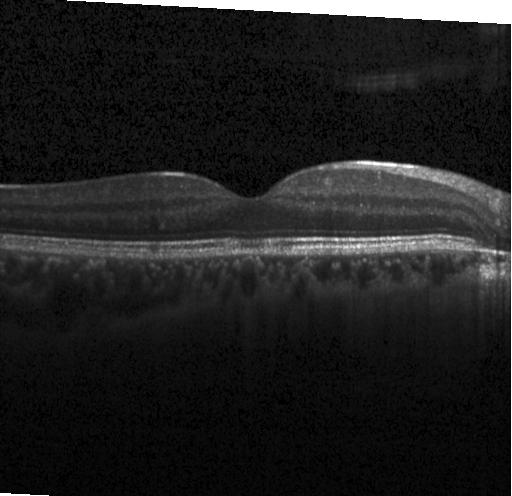

Macular OCT demonstrating neither choroidal neovascularization, diabetic macular edema, nor drusen.